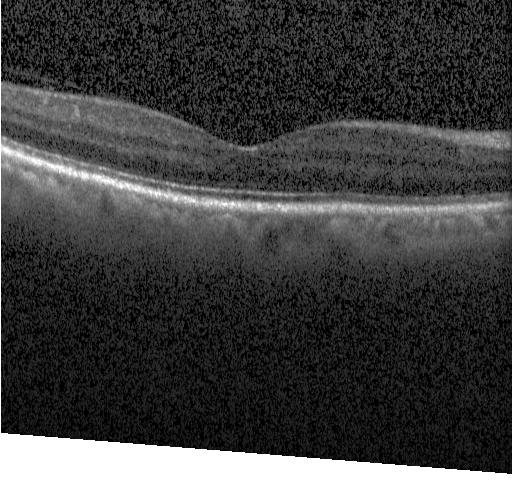
Impression: no evidence of choroidal neovascularization, diabetic macular edema, or drusen.